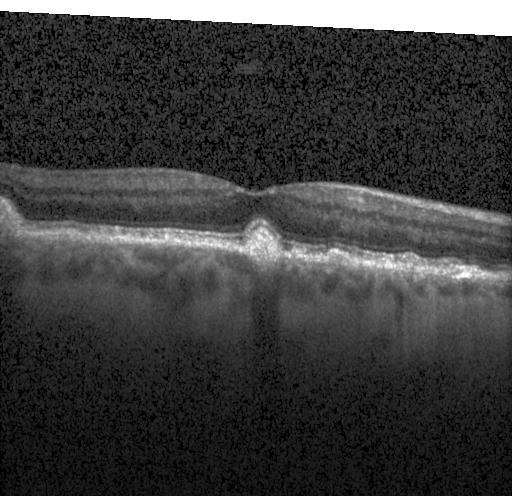 Sub-RPE drusenoid deposits.